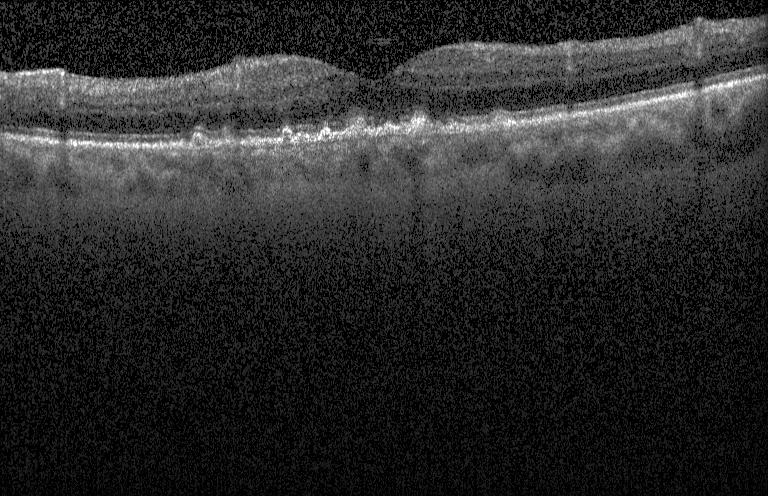

OCT line scan. Instrument: Heidelberg Spectralis. This B-scan demonstrates sub-RPE drusenoid deposits.